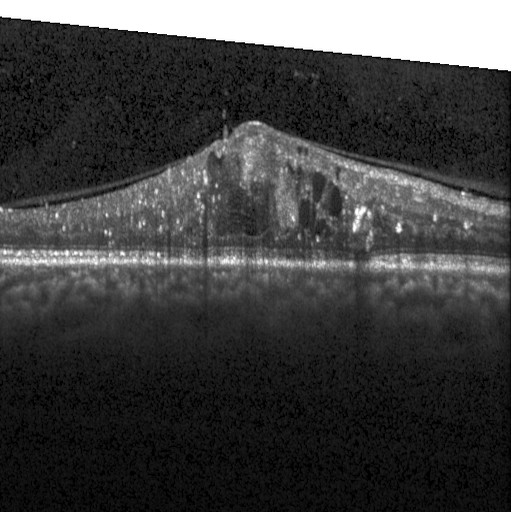
Impression: diabetic macular edema (DME).